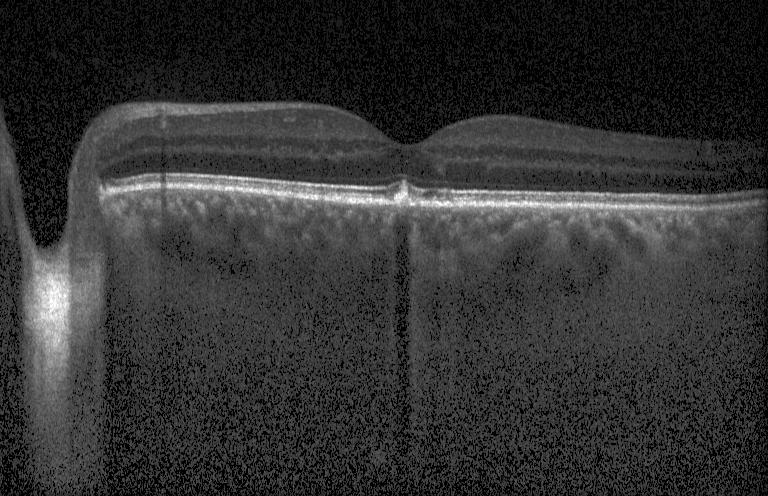 Spectral-domain optical coherence tomography, optical coherence tomography B-scan, Heidelberg Spectralis, centered on the fovea.
This B-scan demonstrates multiple drusen.